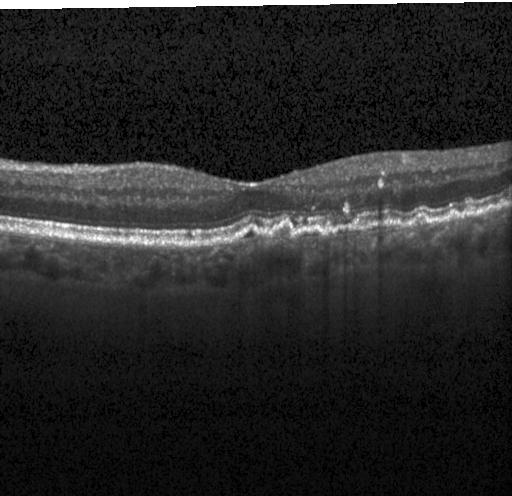 Impression: sub-RPE drusenoid deposits.